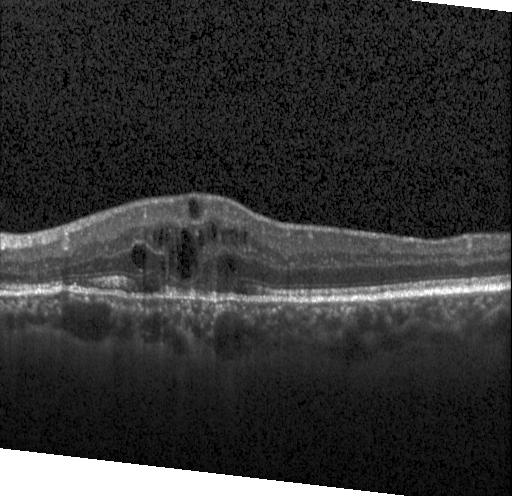
Retinal OCT B-scan. Through the macula.
Diabetic macular edema (DME).